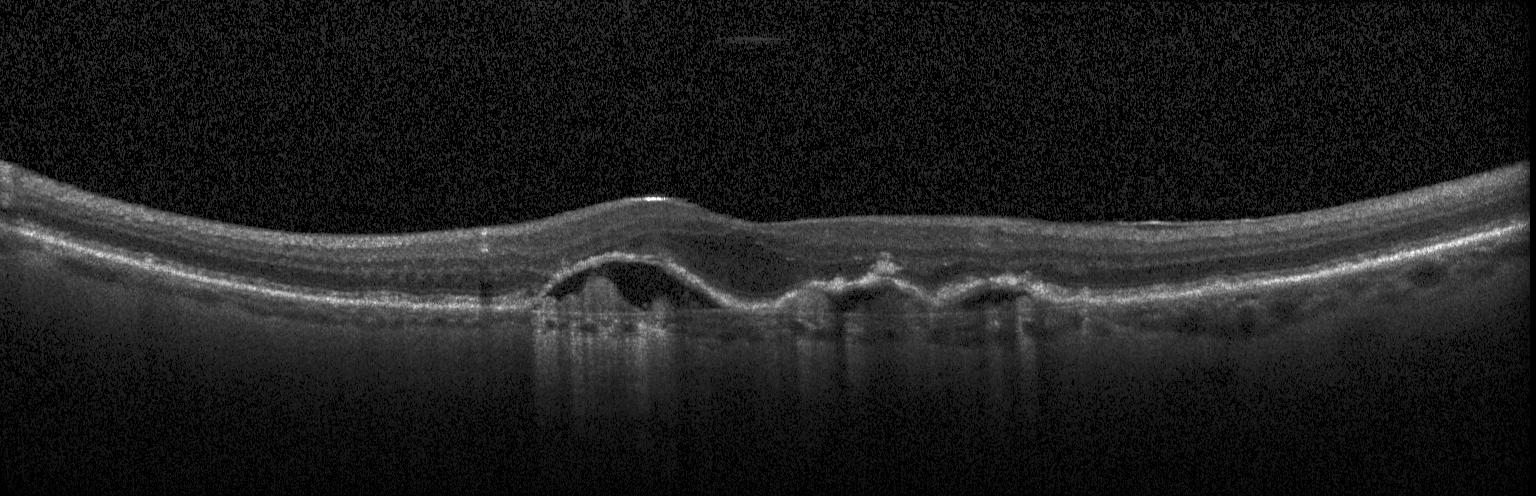
Horizontal scan through the fovea; spectral-domain OCT; OCT line scan.
CNV.